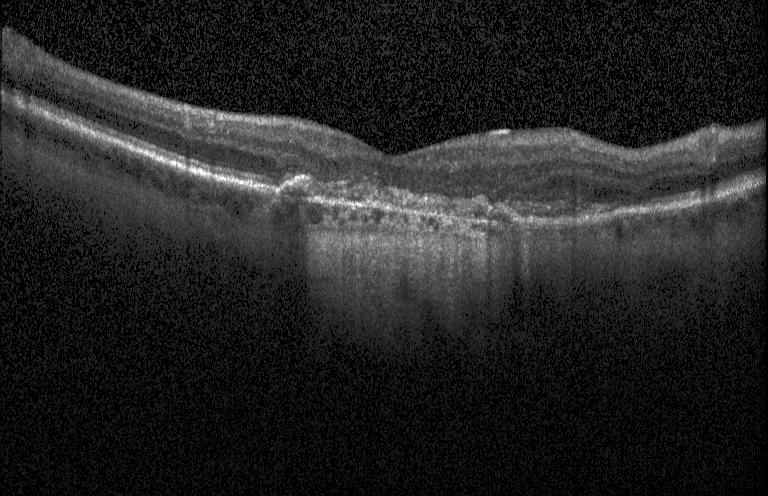
The scan shows a choroidal neovascular membrane.